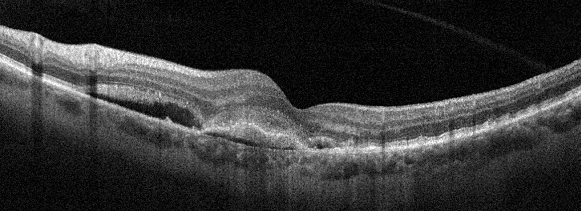
Retinal OCT B-scan · oculus sinister
Impression: AMD.